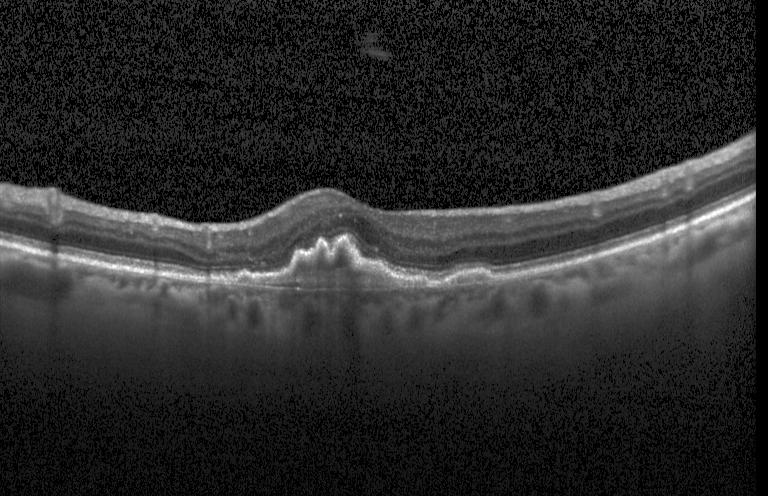
Fovea-centered; optical coherence tomography B-scan.
OCT finding: choroidal neovascularization (CNV).